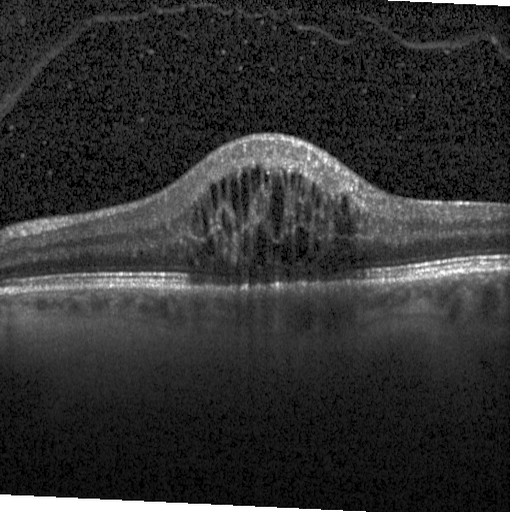

OCT finding: diabetic macular edema.